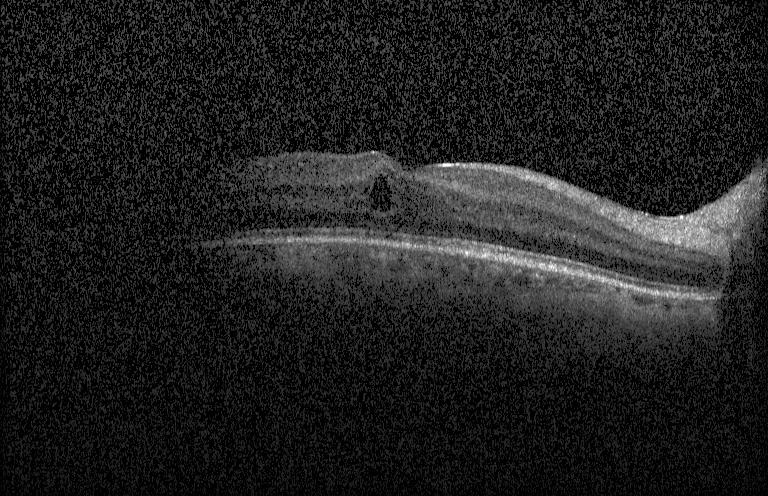
DME.